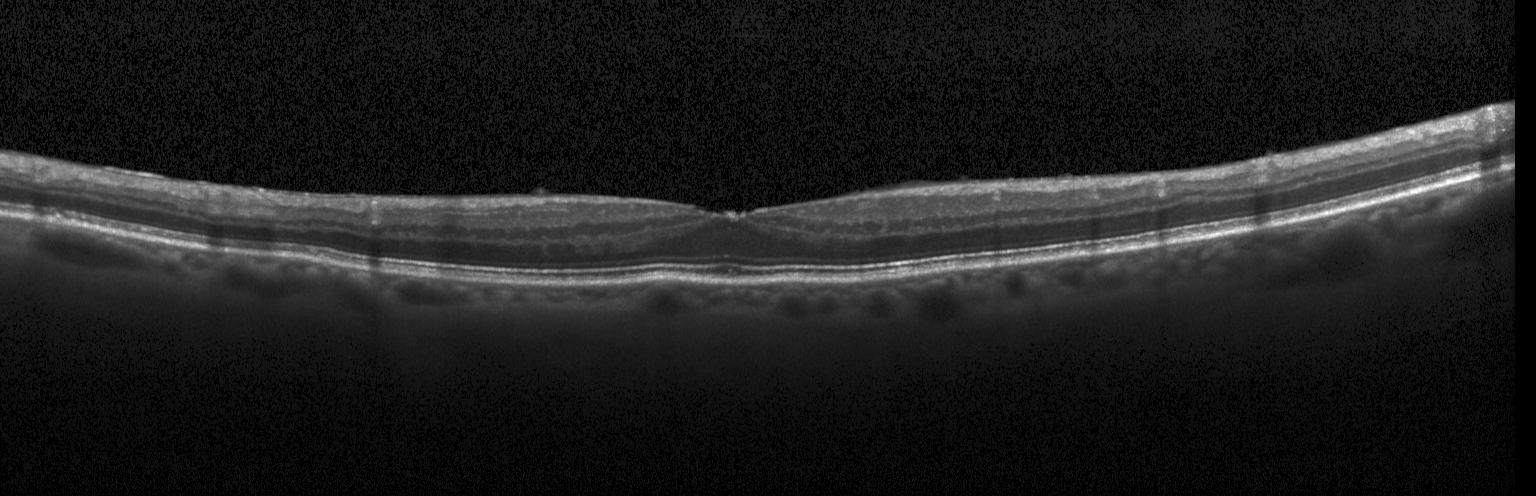 Assessment: neither choroidal neovascularization, diabetic macular edema, nor drusen.